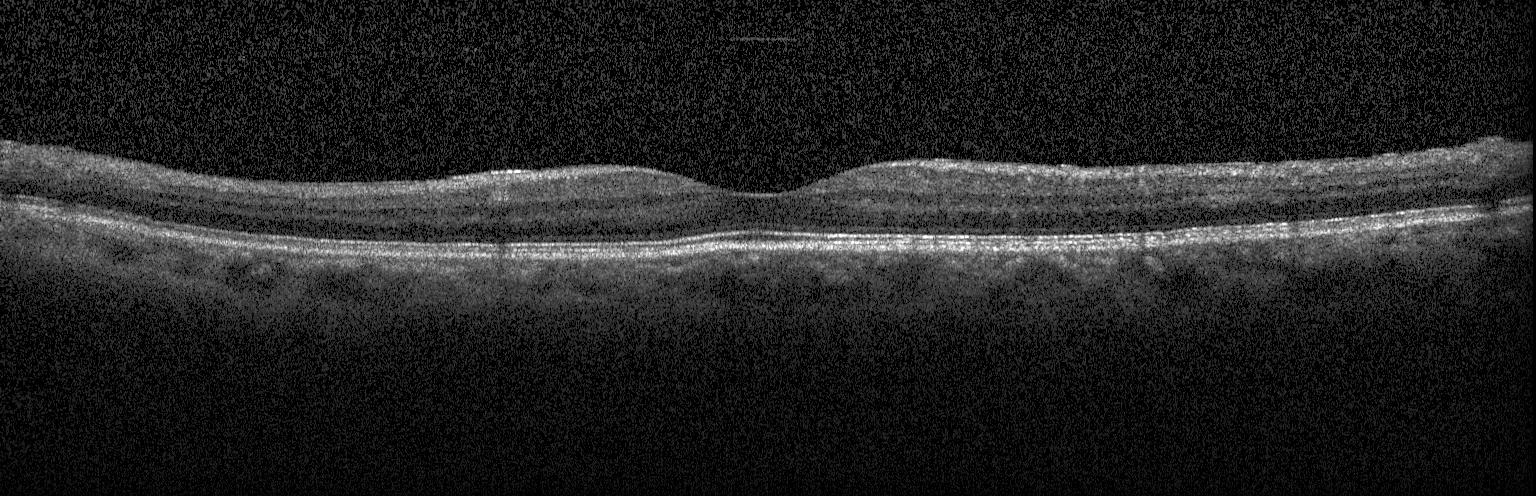

Optical coherence tomography scan. Horizontal scan through the fovea. Spectral-domain OCT.
Finding: no evidence of choroidal neovascularization, diabetic macular edema, or drusen.